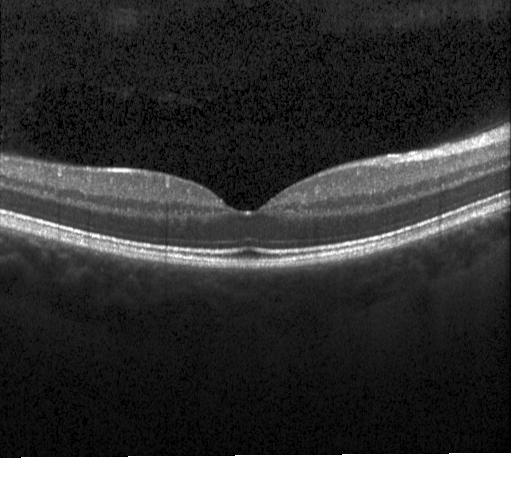
Macular OCT: neither choroidal neovascularization, diabetic macular edema, nor drusen.